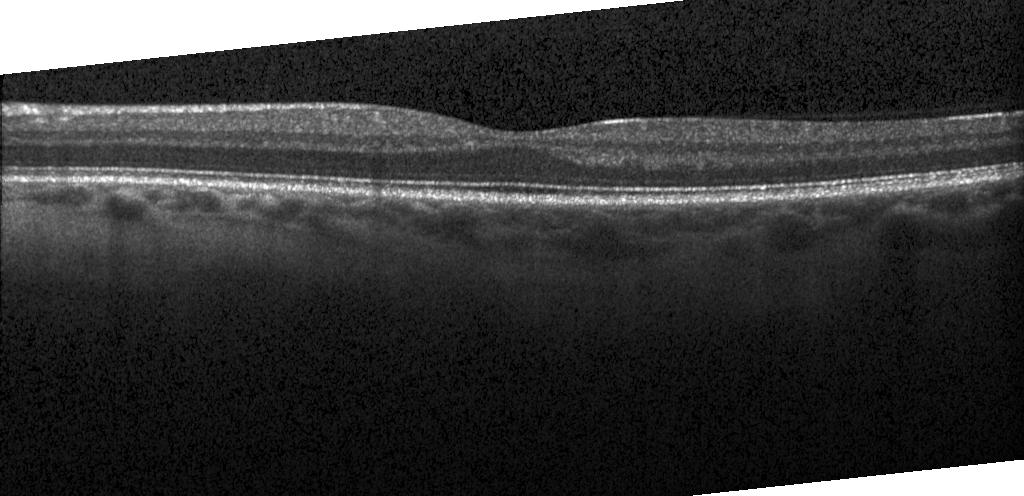

Heidelberg Spectralis · through the macula · retinal OCT cross-section · spectral-domain OCT. OCT finding: no evidence of CNV, DME, or drusen.